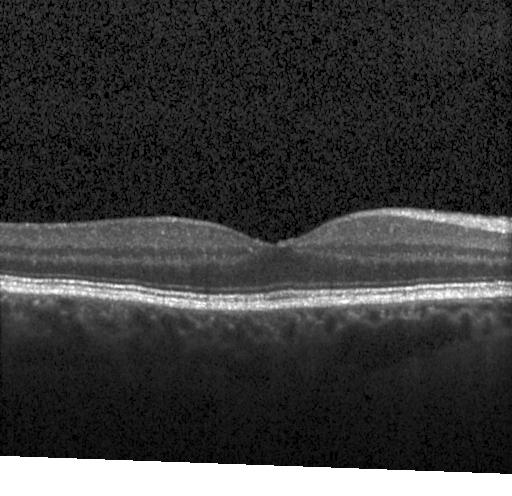 Neither choroidal neovascularization, diabetic macular edema, nor drusen.